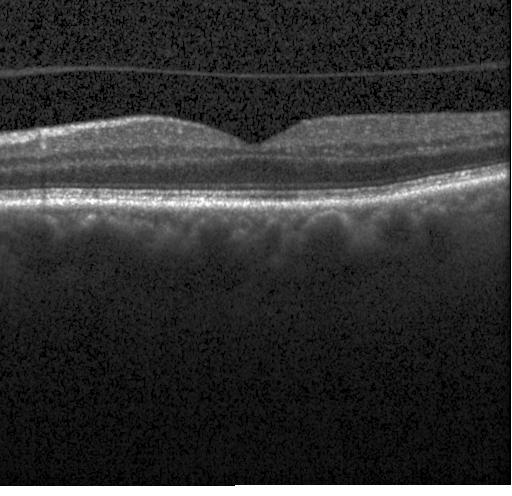
Macular OCT: no choroidal neovascularization, no diabetic macular edema, and no drusen.